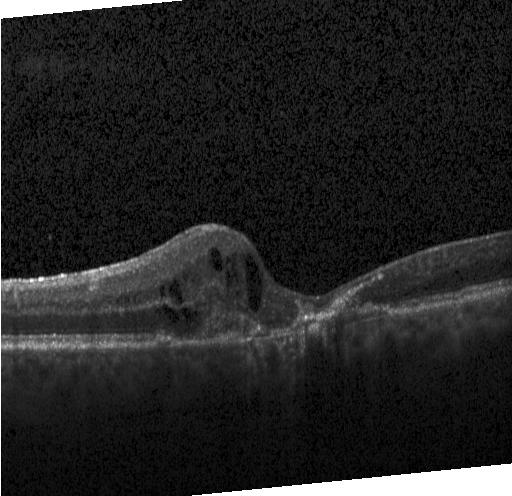 Optical coherence tomography B-scan
OCT finding: choroidal neovascularization.